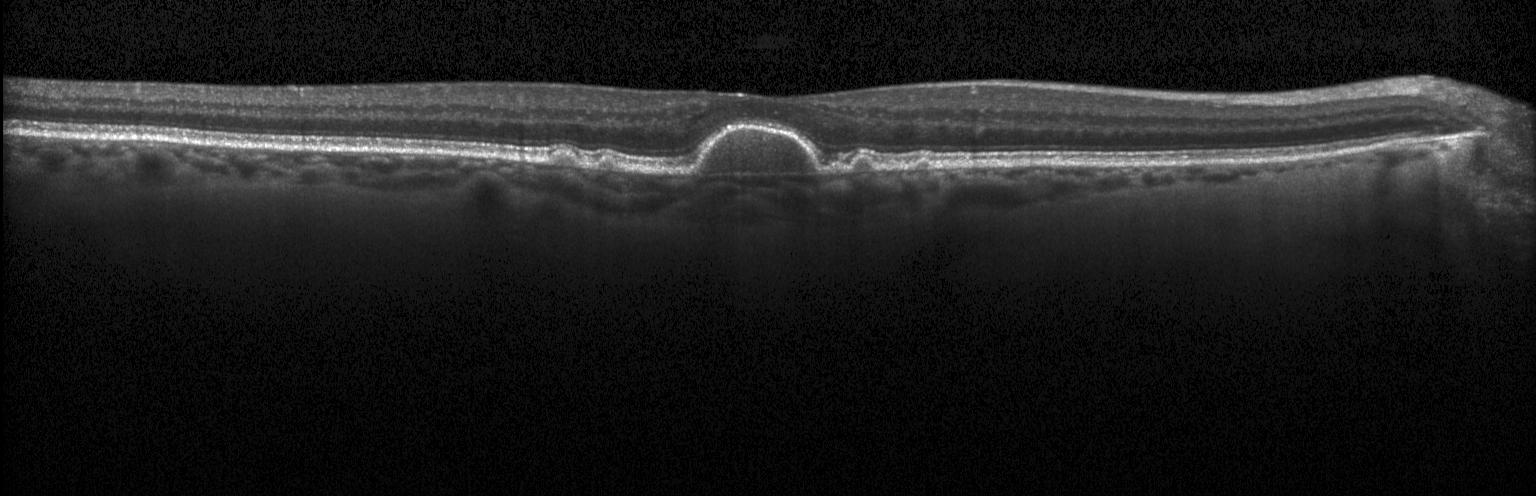 Retinal OCT cross-section, instrument: Heidelberg Spectralis, SD-OCT.
Impression: a choroidal neovascular membrane.